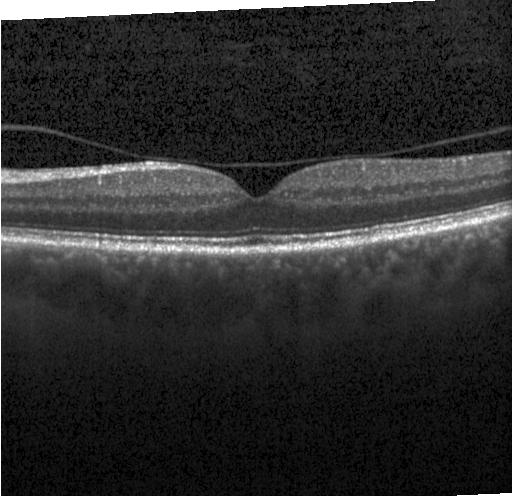 Optical coherence tomography scan; instrument: Heidelberg Spectralis; horizontal scan through the fovea — Diagnosis: no CNV, no DME, and no drusen.